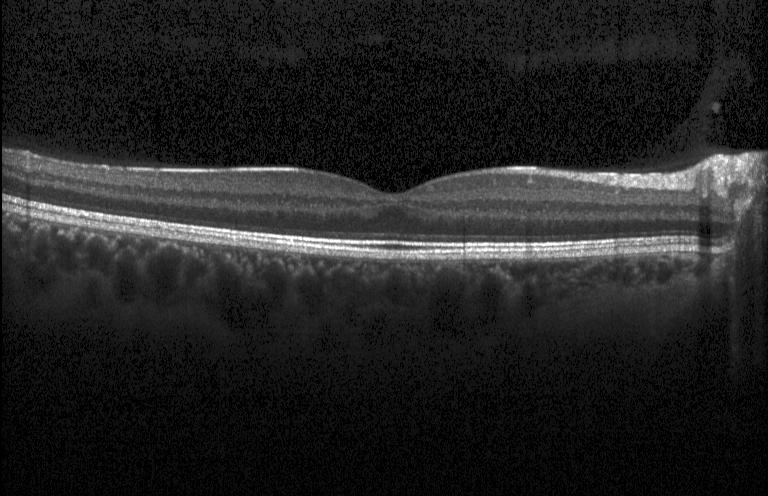

Impression: neither CNV, DME, nor drusen.